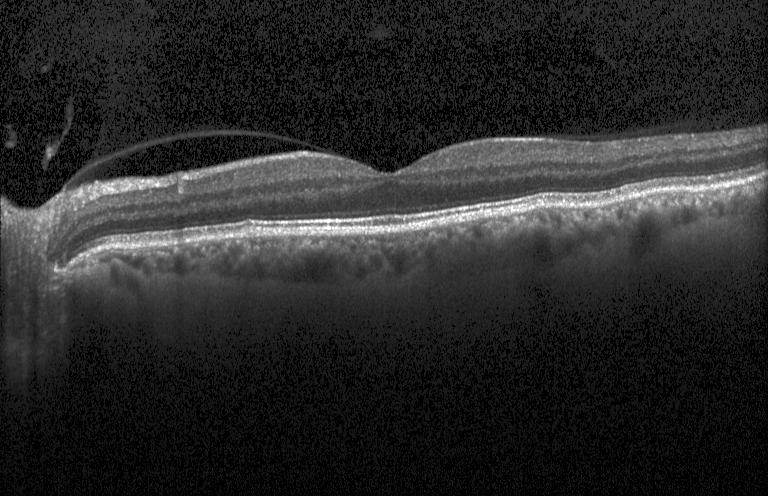 Macular OCT: no choroidal neovascularization, no diabetic macular edema, and no drusen.